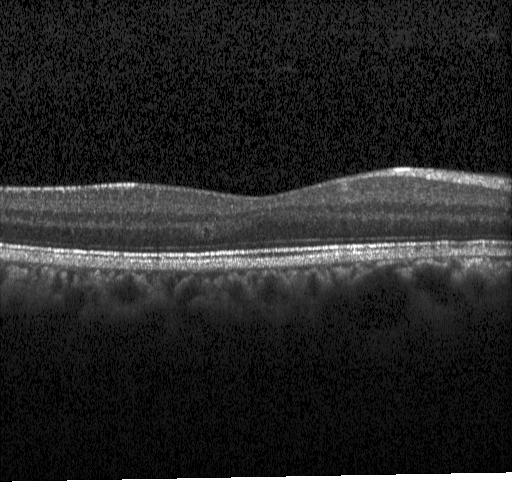

OCT B-scan. Spectral-domain OCT. Macular scan. Heidelberg Spectralis. Impression: no choroidal neovascularization, no diabetic macular edema, and no drusen.